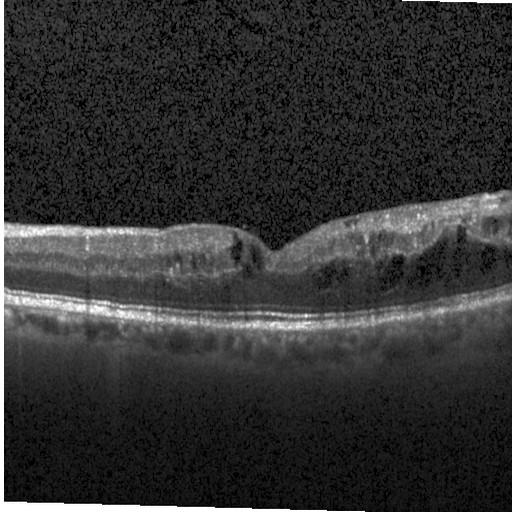 Retinal OCT cross-section · spectral-domain OCT · centered on the fovea — Impression: diabetic macular edema (DME).